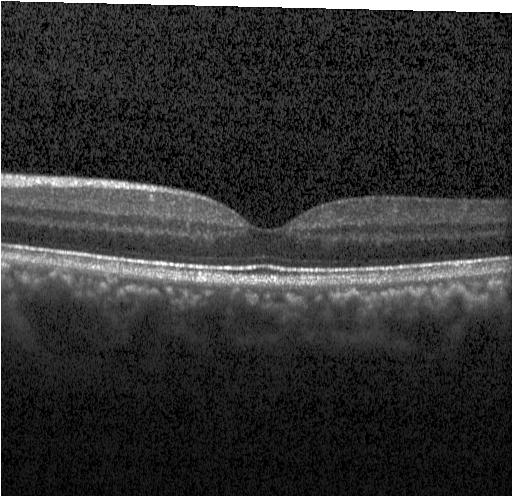 Finding: no choroidal neovascularization, no diabetic macular edema, and no drusen.